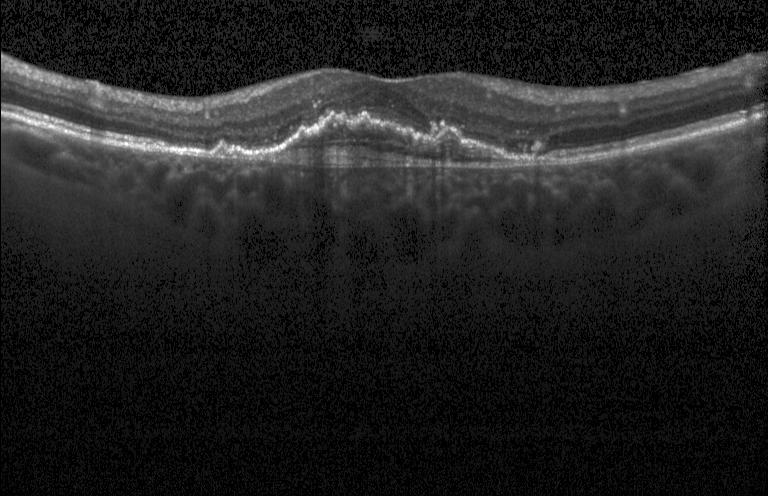
This B-scan demonstrates a choroidal neovascular membrane.